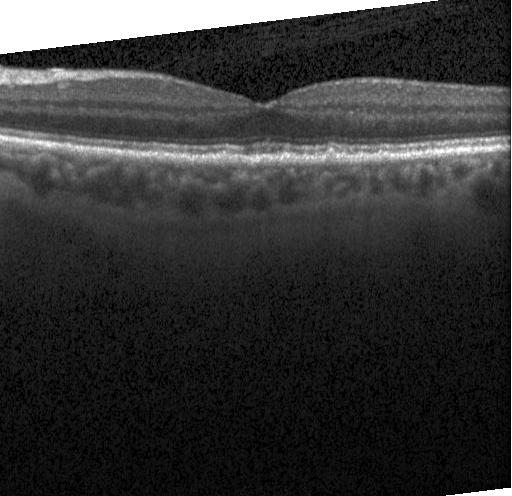 Impression: sub-RPE drusenoid deposits.